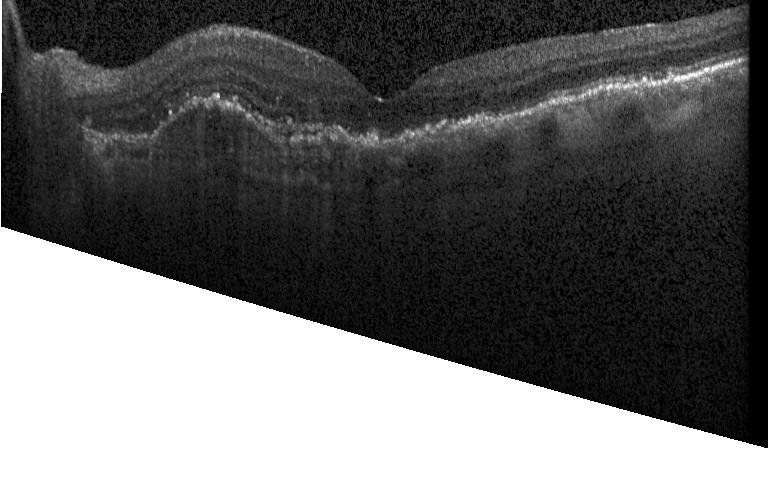
OCT B-scan, SD-OCT — The scan shows choroidal neovascularization.